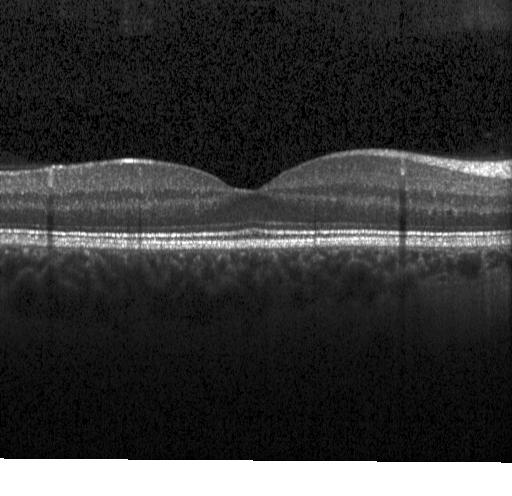
Retinal OCT B-scan — Diagnosis: neither choroidal neovascularization, diabetic macular edema, nor drusen.